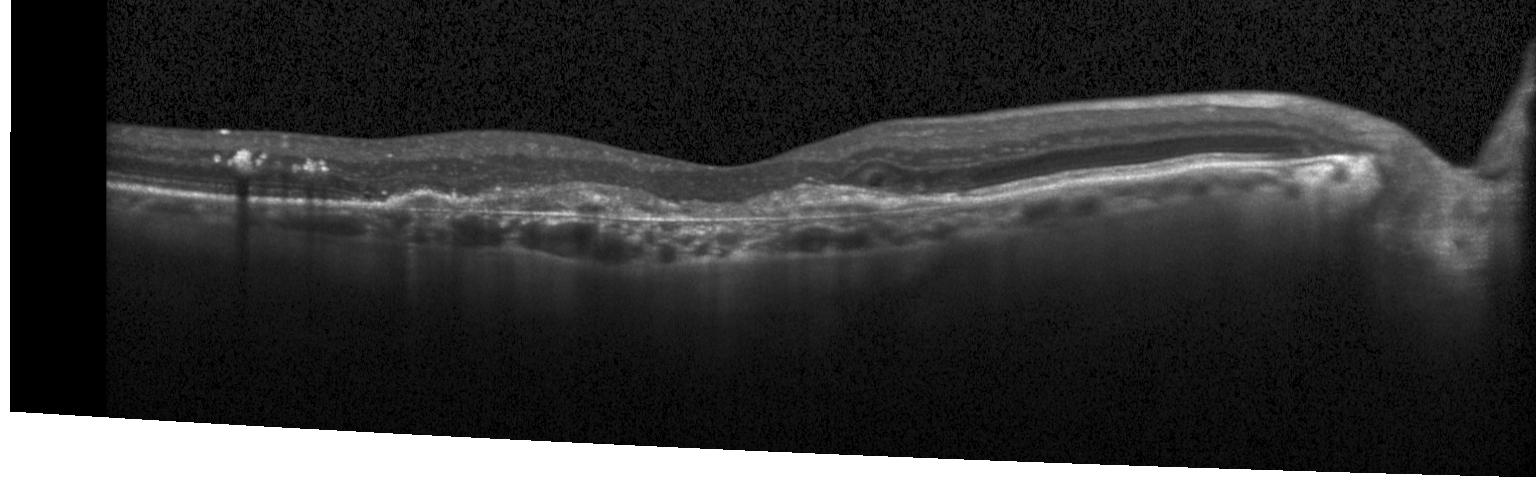 Acquired on a Heidelberg Spectralis, horizontal scan through the fovea, spectral-domain optical coherence tomography, OCT line scan.
Choroidal neovascularization.